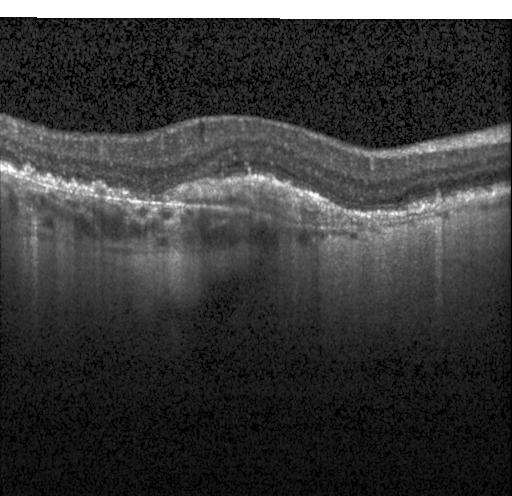 Finding: CNV.